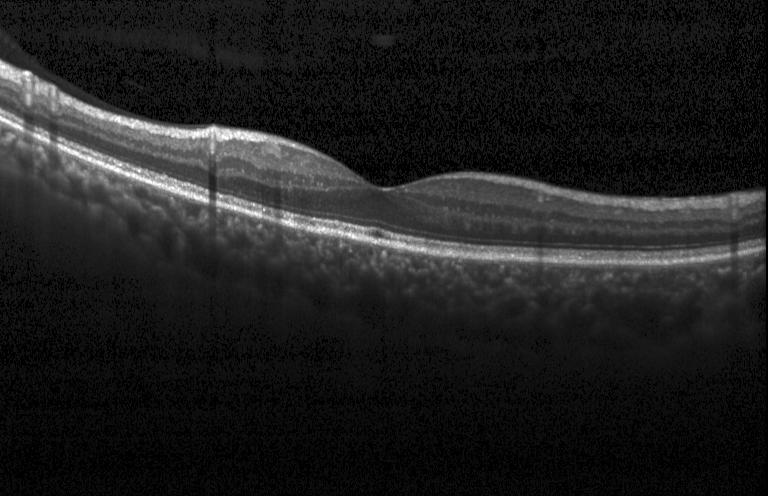 Macular scan · acquired on a Heidelberg Spectralis · optical coherence tomography B-scan · spectral-domain optical coherence tomography. Finding: no choroidal neovascularization, no diabetic macular edema, and no drusen.